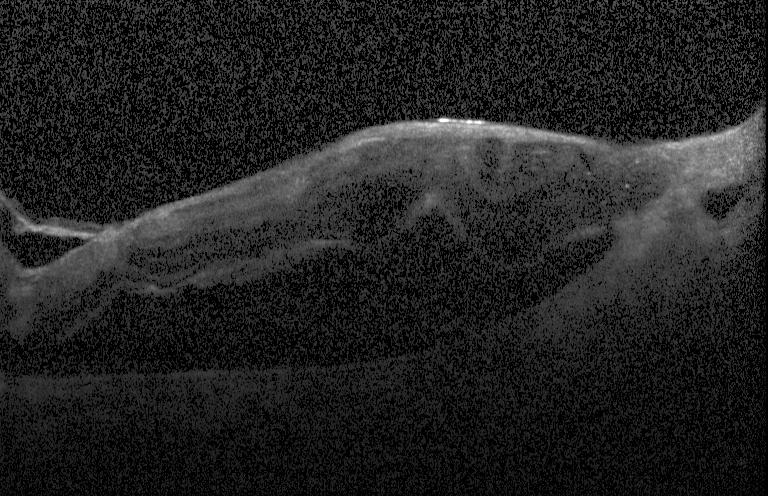

Diagnosis: diabetic macular edema (DME).